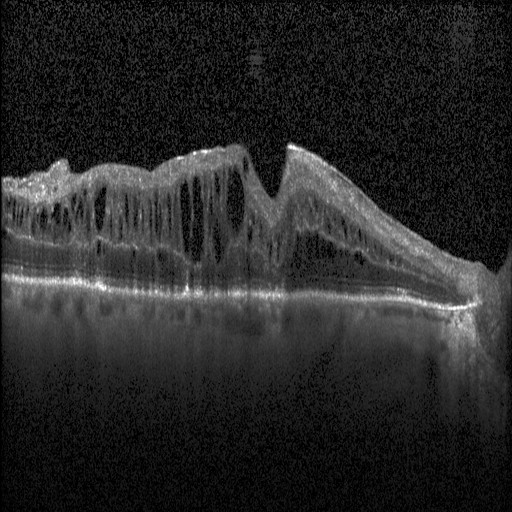
Horizontal scan through the fovea. OCT line scan.
Dx: DME.